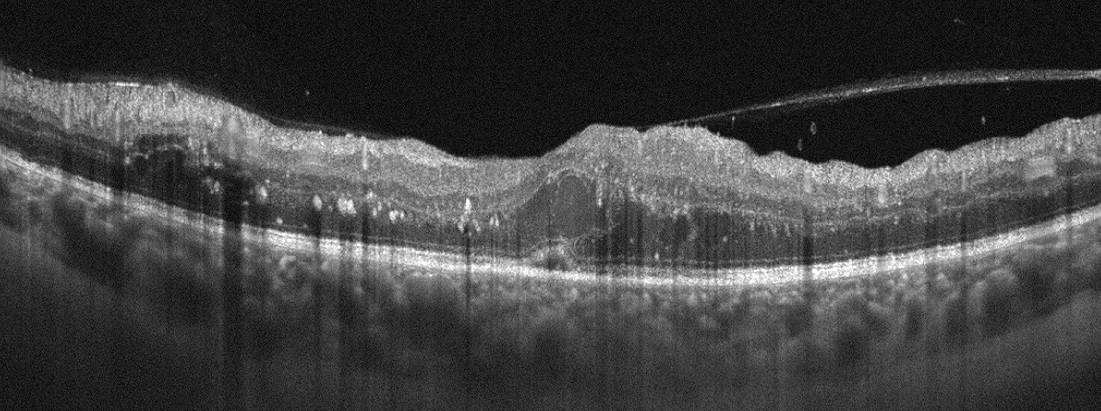 Optical coherence tomography scan — Diagnosis: diabetic macular edema.